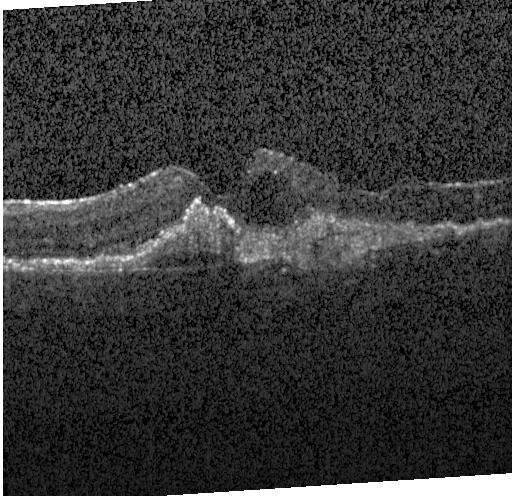 Horizontal scan through the fovea · SD-OCT · retinal OCT B-scan · instrument: Heidelberg Spectralis.
Finding: choroidal neovascularization (CNV).